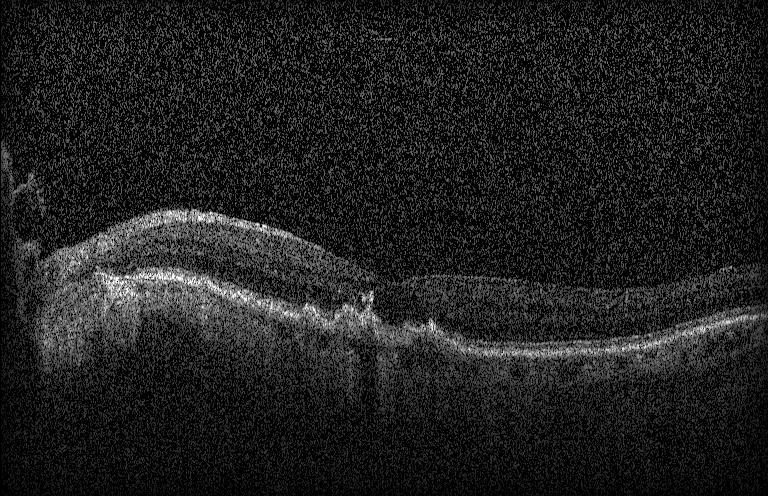 Horizontal scan through the fovea · OCT line scan · spectral-domain optical coherence tomography.
Dx: sub-RPE drusenoid deposits.